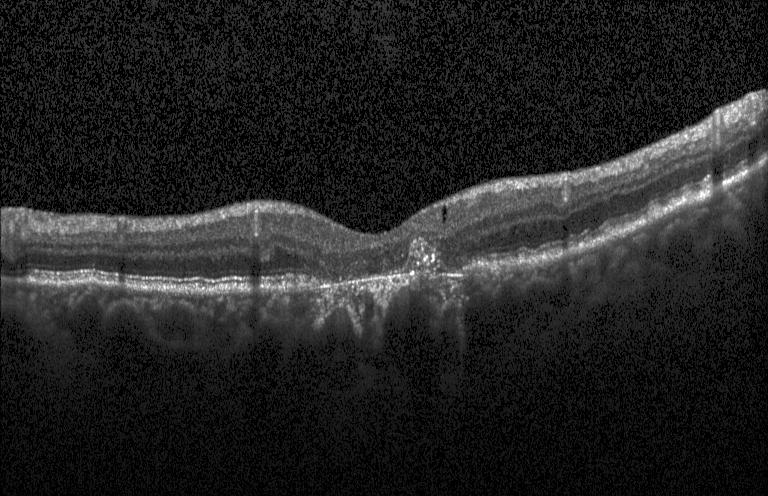 OCT finding: choroidal neovascularization.